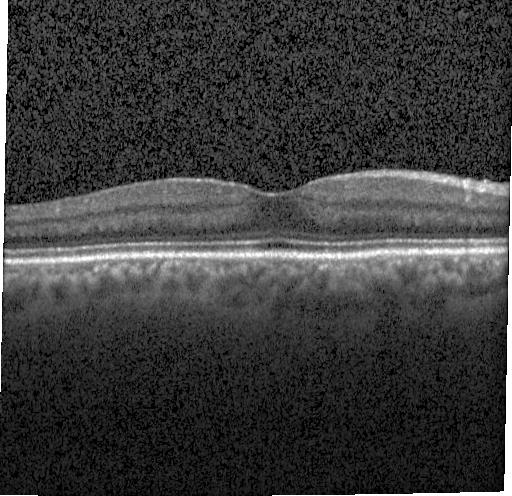

Macular OCT: no choroidal neovascularization, no diabetic macular edema, and no drusen.